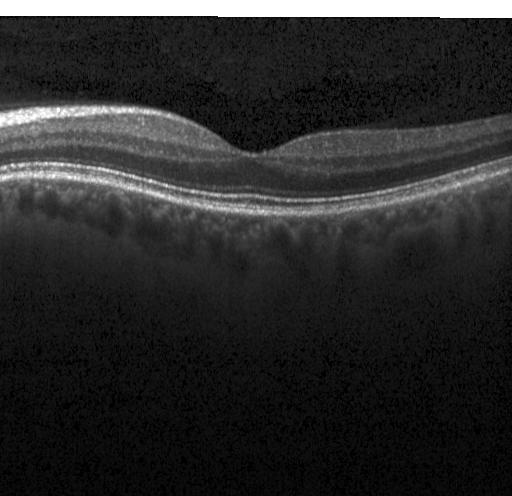
OCT scan showing no choroidal neovascularization, diabetic macular edema, or drusen.